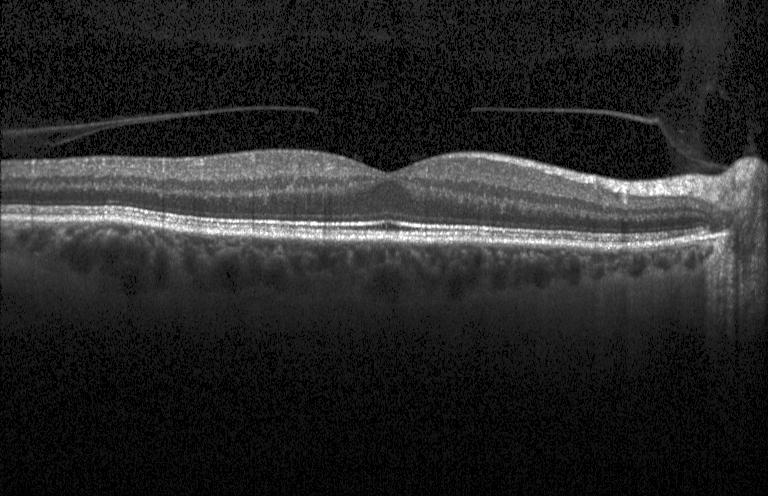
OCT scan showing no CNV, DME, or drusen.